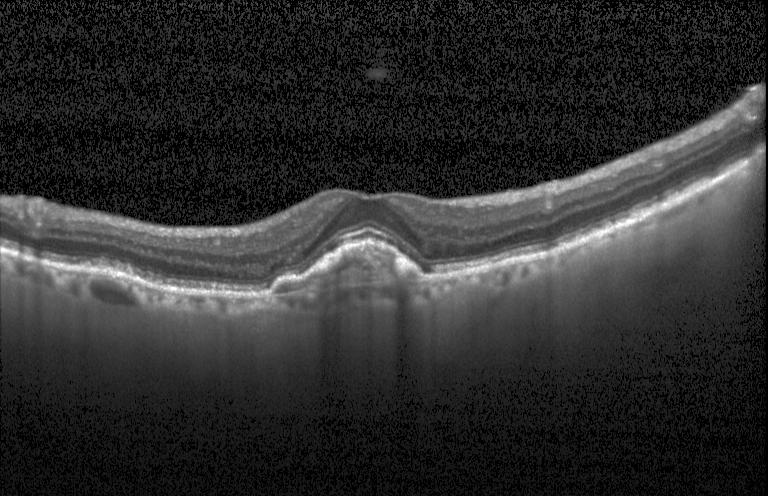

OCT line scan.
Impression: choroidal neovascularization.